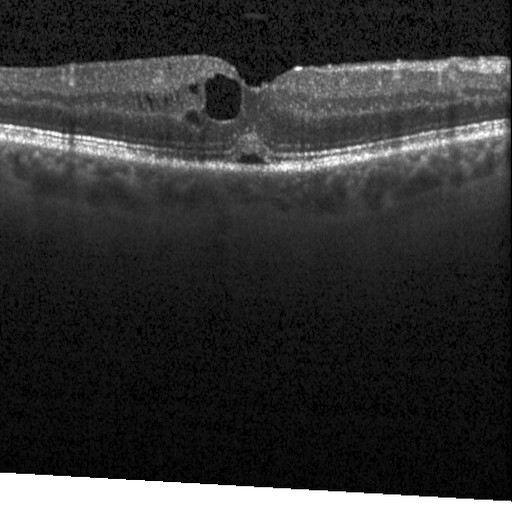
Fovea-centered; SD-OCT; OCT B-scan; Heidelberg Spectralis
Macular OCT: DME.